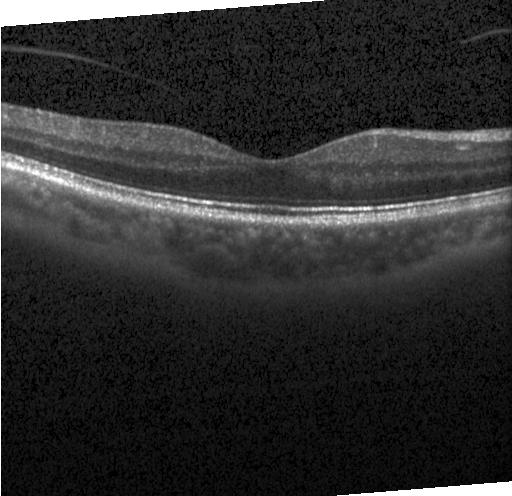

Fovea-centered · OCT B-scan · Heidelberg Spectralis OCT system · SD-OCT
Finding: neither choroidal neovascularization, diabetic macular edema, nor drusen.